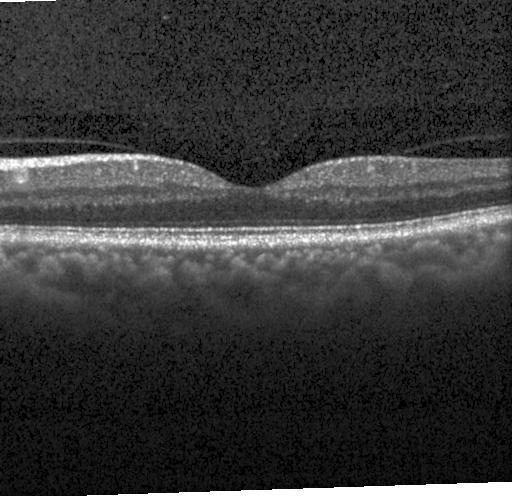

Horizontal scan through the fovea · optical coherence tomography scan
Finding: no evidence of CNV, DME, or drusen.